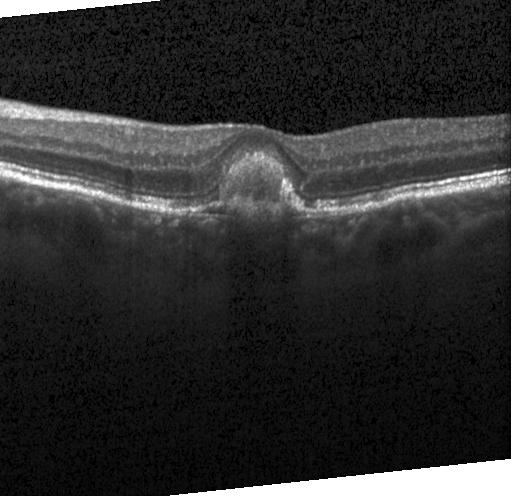
Diagnosis: a choroidal neovascular membrane.